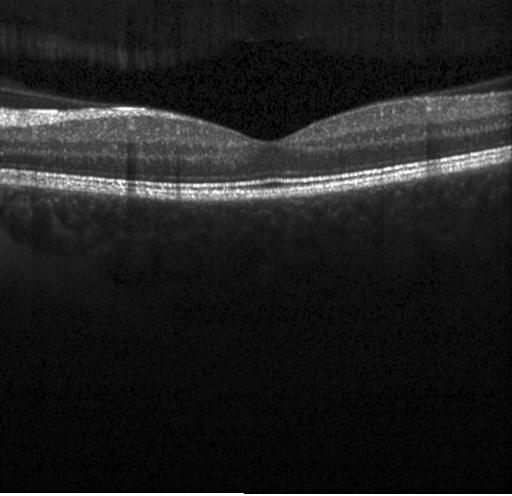 Retinal OCT cross-section showing no CNV, DME, or drusen.